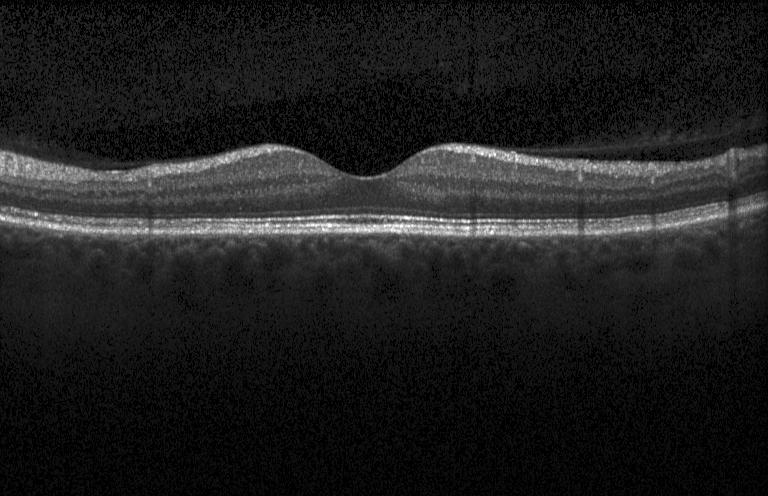 Horizontal scan through the fovea; Heidelberg Spectralis; optical coherence tomography B-scan; SD-OCT.
The scan shows no choroidal neovascularization, no diabetic macular edema, and no drusen.